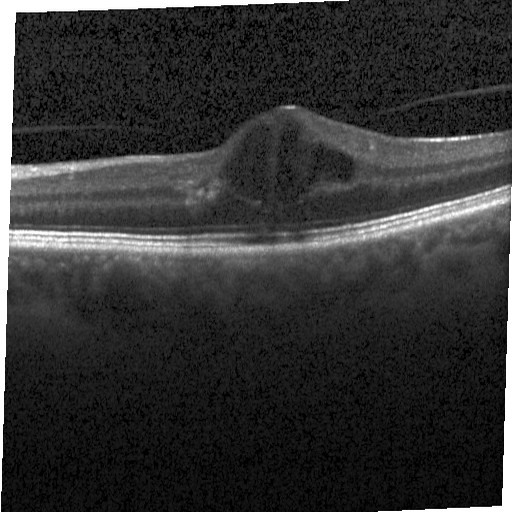

Spectral-domain OCT. Optical coherence tomography scan. Instrument: Heidelberg Spectralis.
The scan shows DME.